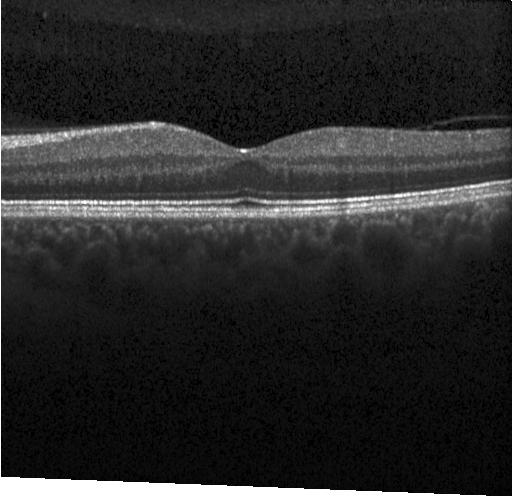 Diagnosis: no choroidal neovascularization, diabetic macular edema, or drusen.